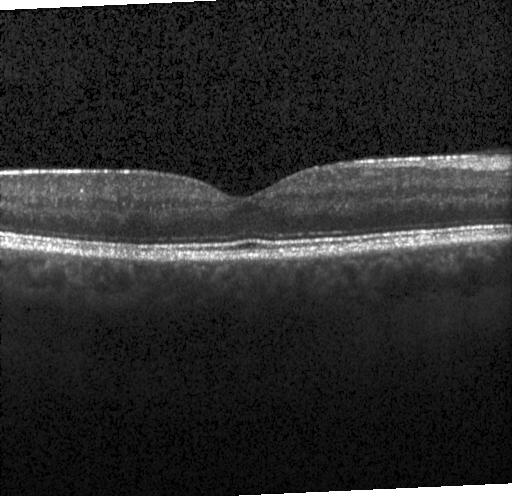 Optical coherence tomography scan. Acquired on a Heidelberg Spectralis — Assessment: no CNV, DME, or drusen.